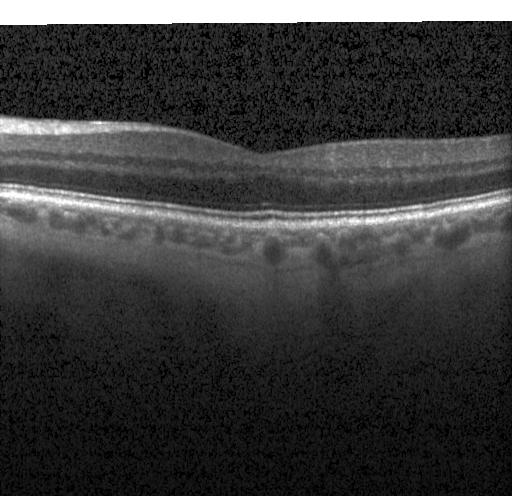

Centered on the fovea; spectral-domain OCT; optical coherence tomography B-scan. Macular OCT: neither CNV, DME, nor drusen.